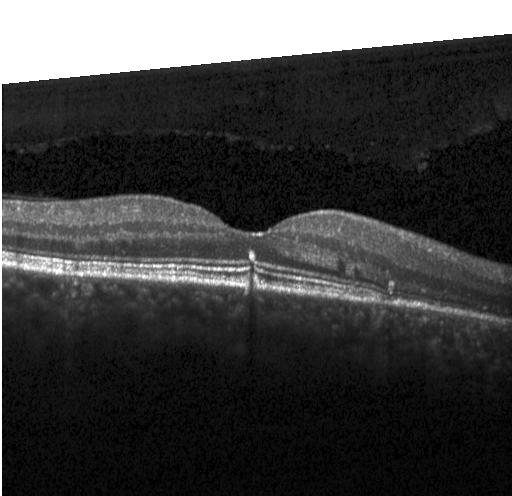 Optical coherence tomography B-scan, spectral-domain optical coherence tomography. OCT finding: sub-RPE drusenoid deposits.